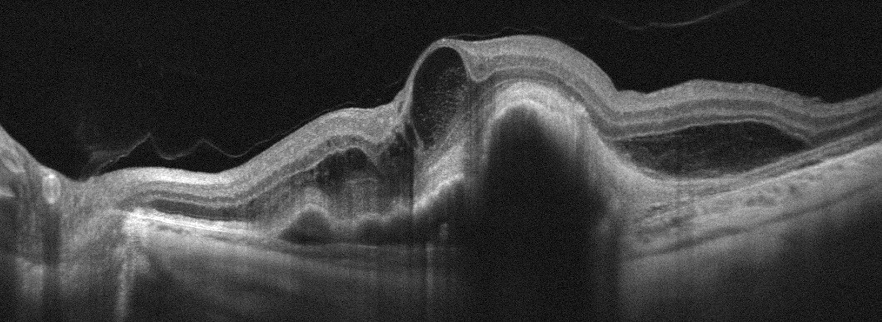

Fovea-centered, instrument: Optovue Avanti RTVue XR, OCT B-scan. OCT finding: age-related macular degeneration.